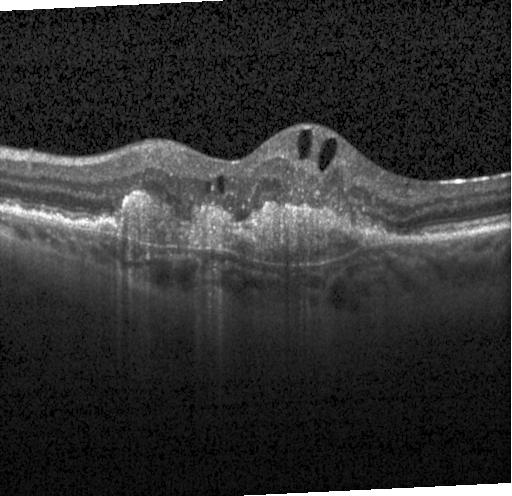
Diagnosis: a choroidal neovascular membrane.